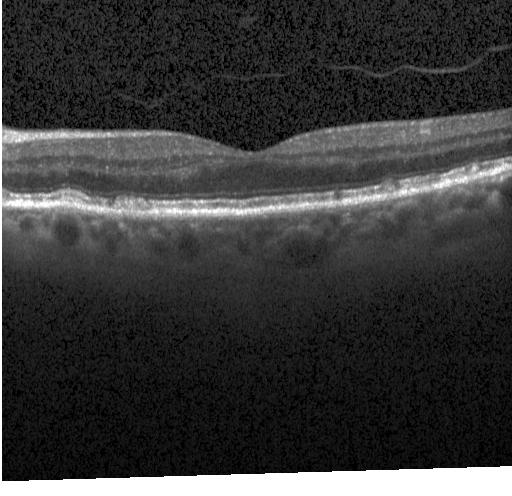
Fovea-centered; spectral-domain OCT; acquired on a Heidelberg Spectralis; optical coherence tomography scan. Diagnosis: sub-RPE drusenoid deposits.